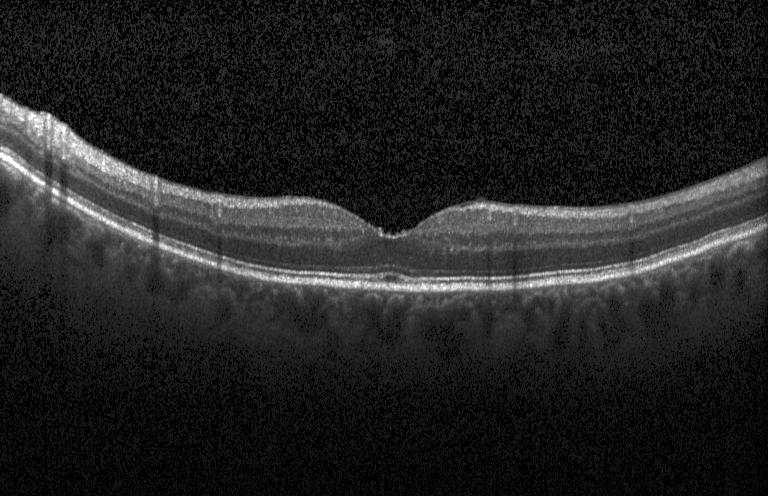
Spectral-domain OCT. Through the macula. Heidelberg Spectralis. Retinal OCT cross-section.
The scan shows neither choroidal neovascularization, diabetic macular edema, nor drusen.